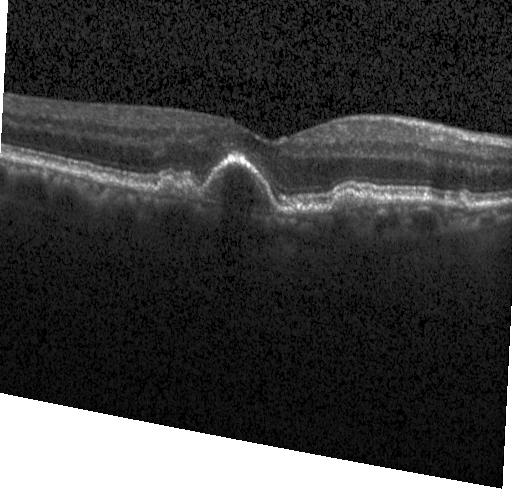
Finding: drusen.